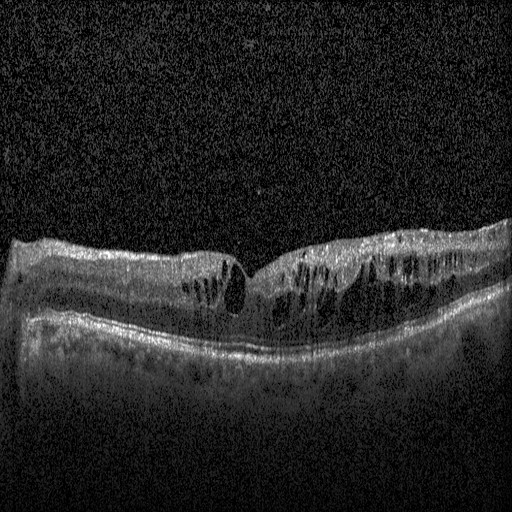 Heidelberg Spectralis. Macular scan. SD-OCT. OCT line scan — Macular OCT: diabetic macular edema.